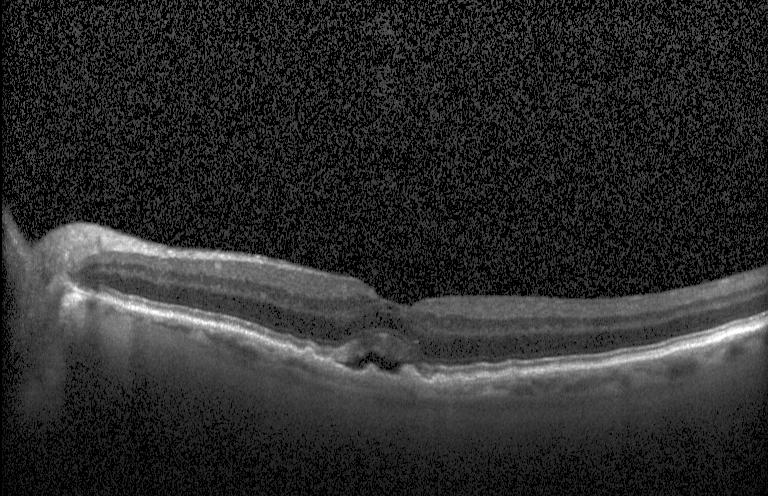

Spectral-domain OCT. Heidelberg Spectralis. Fovea-centered. Optical coherence tomography scan
Dx: a choroidal neovascular membrane.